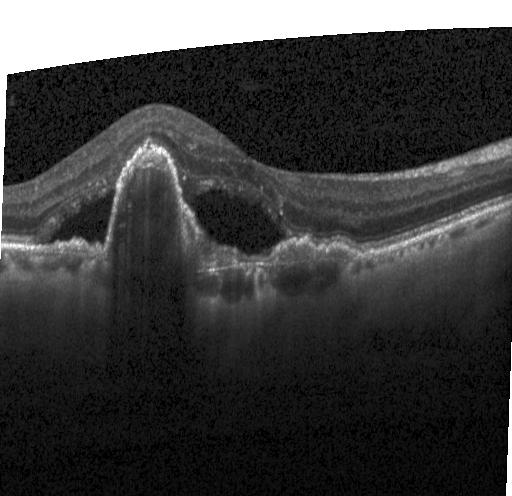
Diagnosis: choroidal neovascularization (CNV).